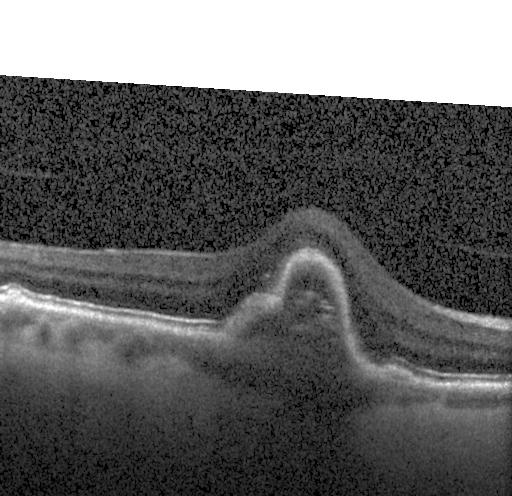
Retinal OCT cross-section. Centered on the fovea. Heidelberg Spectralis OCT system. SD-OCT. Assessment: choroidal neovascularization.